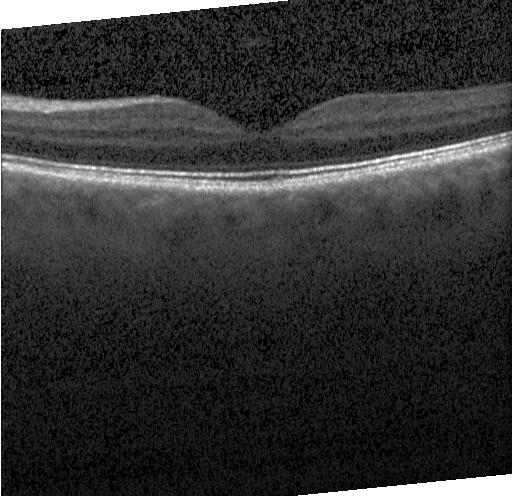
OCT line scan. Macular scan. Finding: neither CNV, DME, nor drusen.